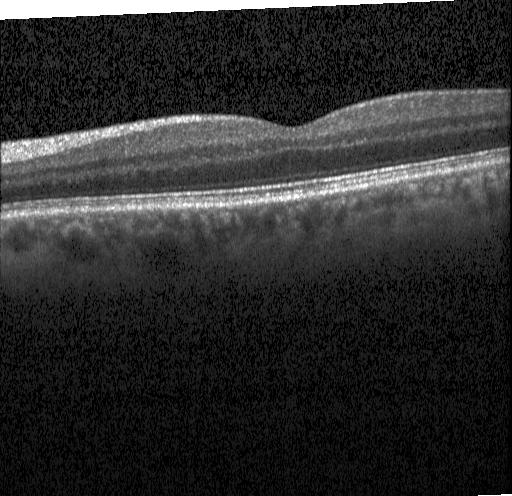

Retinal OCT cross-section.
Impression: no evidence of CNV, DME, or drusen.